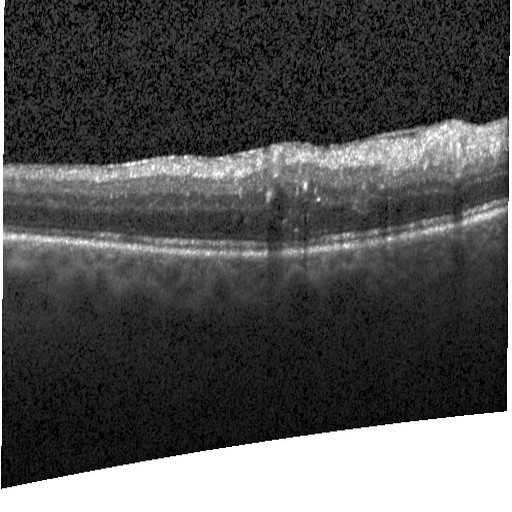
Diagnosis: DME.